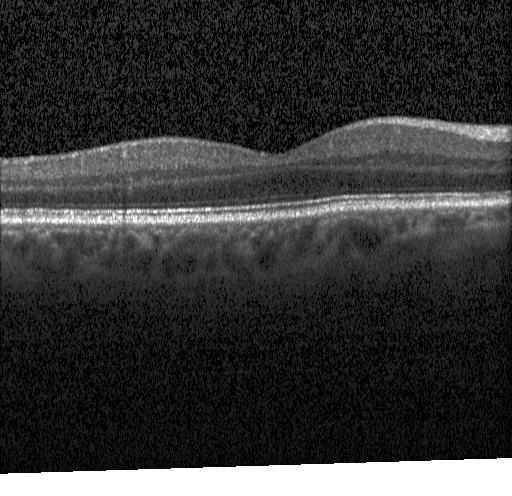

Heidelberg Spectralis OCT system. Through the macula. Spectral-domain OCT. Retinal OCT cross-section. Finding: no evidence of CNV, DME, or drusen.